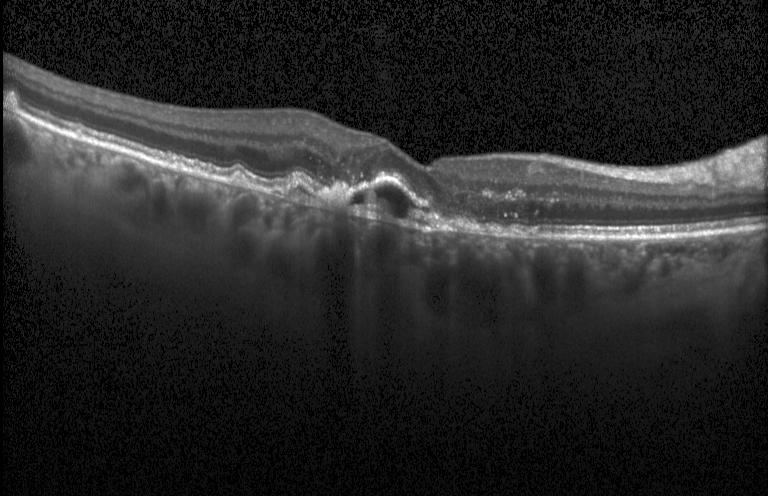
Horizontal scan through the fovea, retinal OCT B-scan. Dx: a choroidal neovascular membrane.